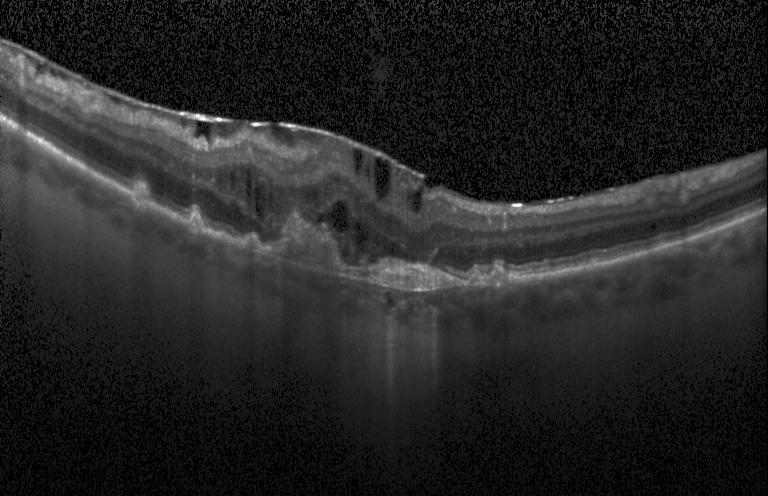 Retinal OCT cross-section; spectral-domain optical coherence tomography; through the macula; instrument: Heidelberg Spectralis
Diagnosis: a choroidal neovascular membrane.